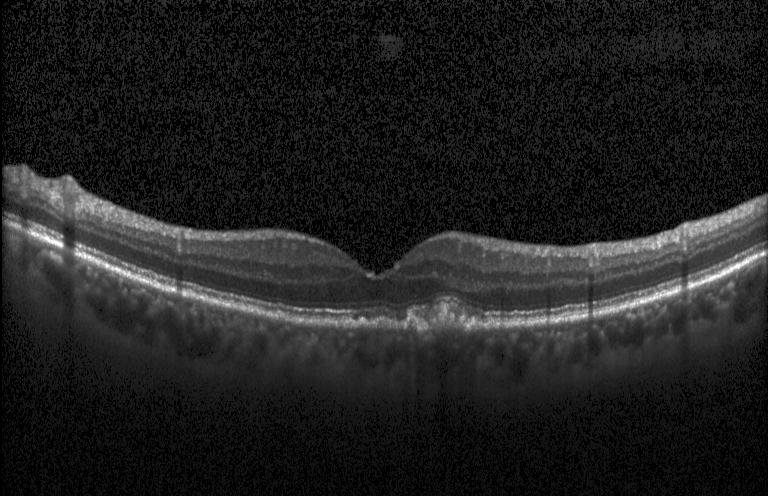 Heidelberg Spectralis; centered on the fovea; optical coherence tomography B-scan; spectral-domain optical coherence tomography
Drusen.